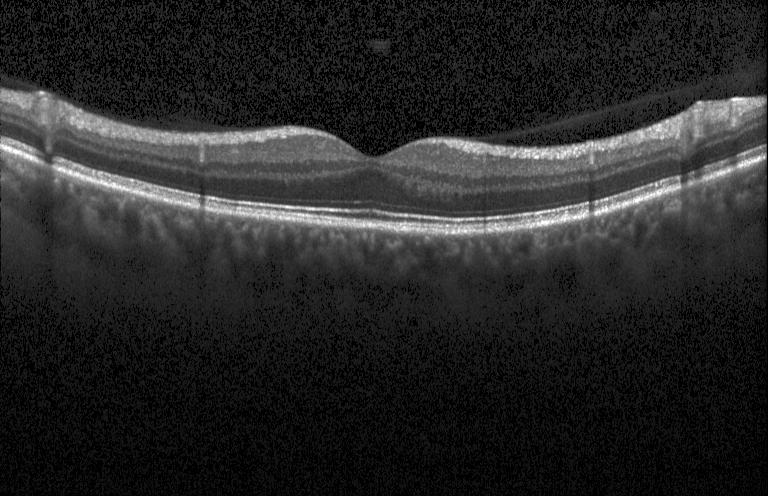 SD-OCT; horizontal scan through the fovea; optical coherence tomography scan; instrument: Heidelberg Spectralis.
Diagnosis: neither choroidal neovascularization, diabetic macular edema, nor drusen.